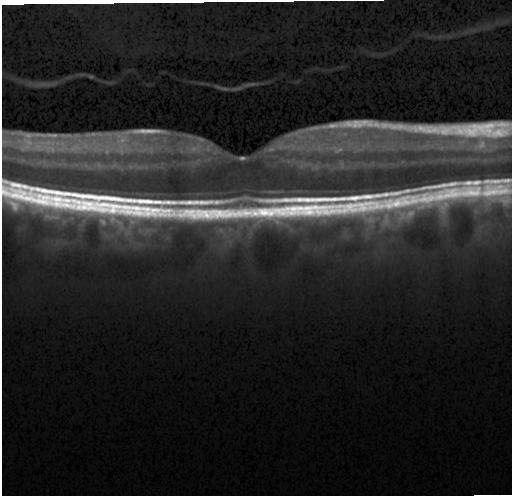 Heidelberg Spectralis; retinal OCT cross-section; through the macula
Finding: no evidence of CNV, DME, or drusen.